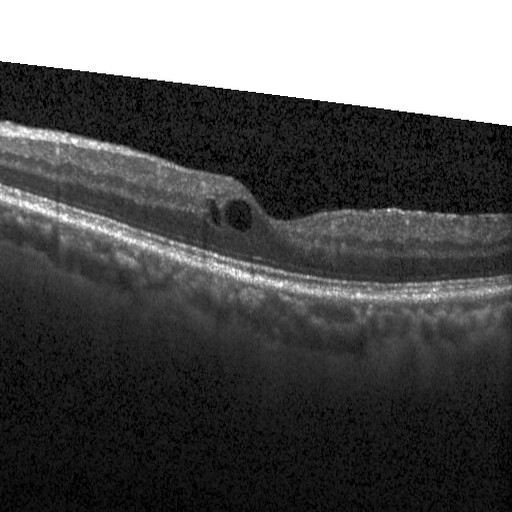
OCT B-scan, spectral-domain OCT — Finding: diabetic macular edema (DME).